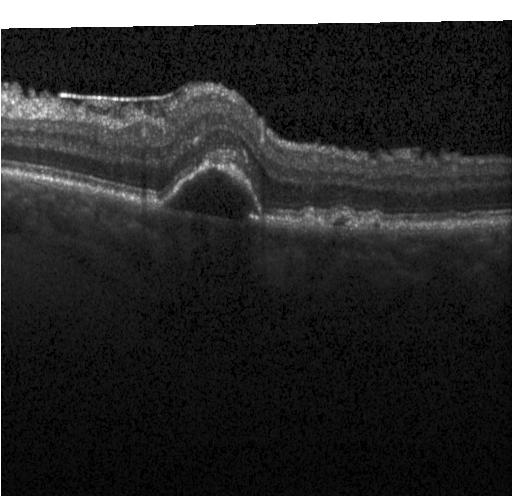
Acquired on a Heidelberg Spectralis, spectral-domain optical coherence tomography, OCT B-scan, centered on the fovea. Diagnosis: a choroidal neovascular membrane.